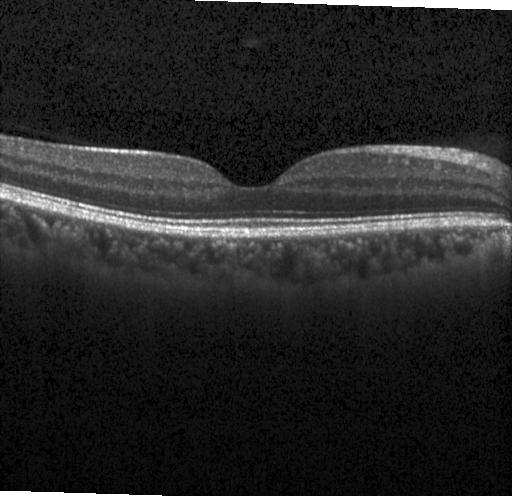
Assessment: no choroidal neovascularization, diabetic macular edema, or drusen.